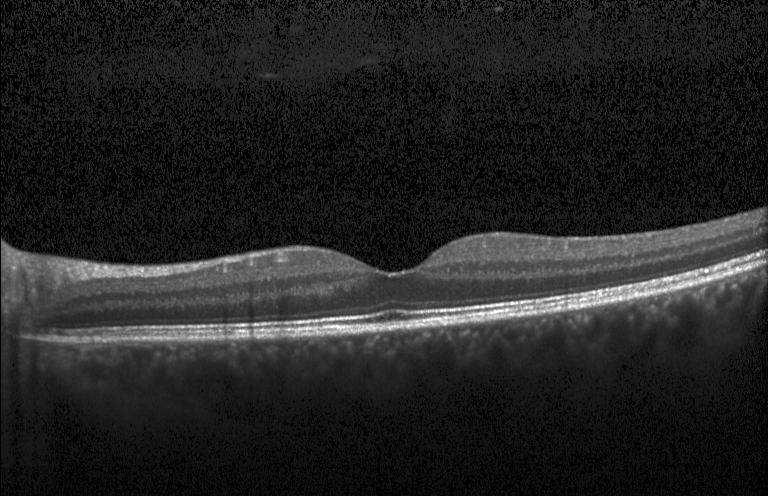 The scan shows no evidence of choroidal neovascularization, diabetic macular edema, or drusen.